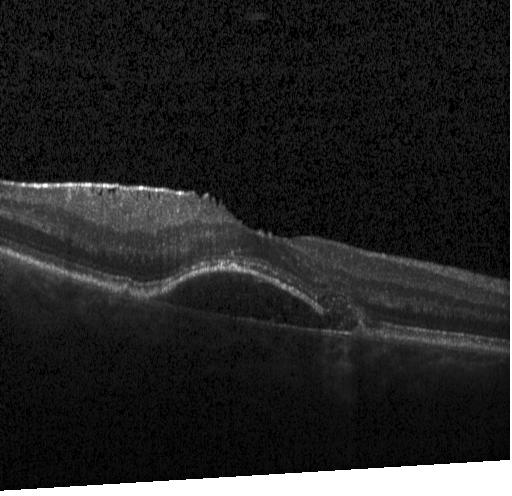
This B-scan demonstrates a choroidal neovascular membrane.